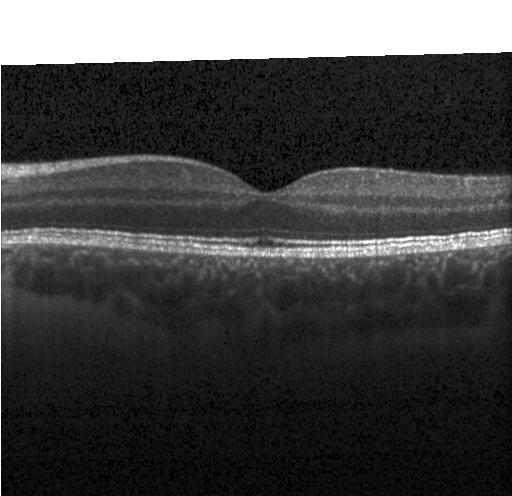

Retinal OCT B-scan
Assessment: no evidence of CNV, DME, or drusen.